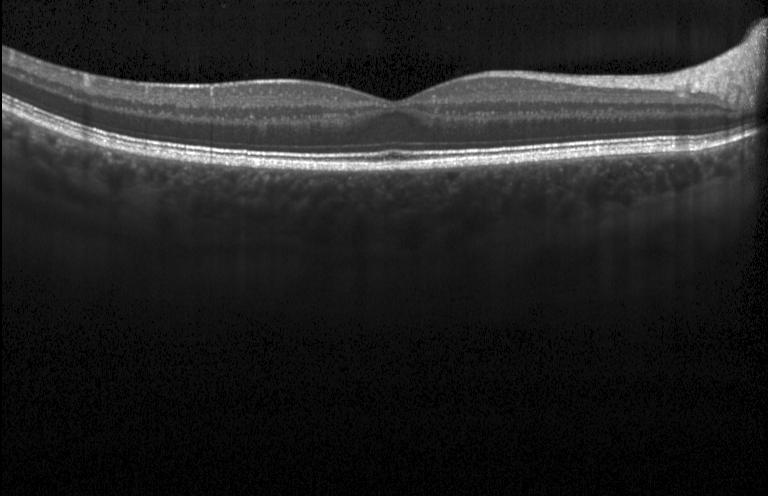 Retinal OCT cross-section, through the macula, Heidelberg Spectralis, SD-OCT — Dx: no choroidal neovascularization, no diabetic macular edema, and no drusen.